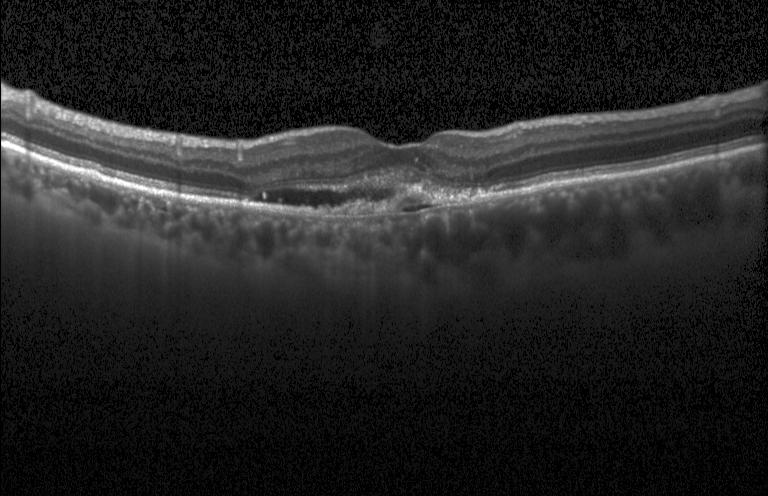
Dx: a choroidal neovascular membrane.